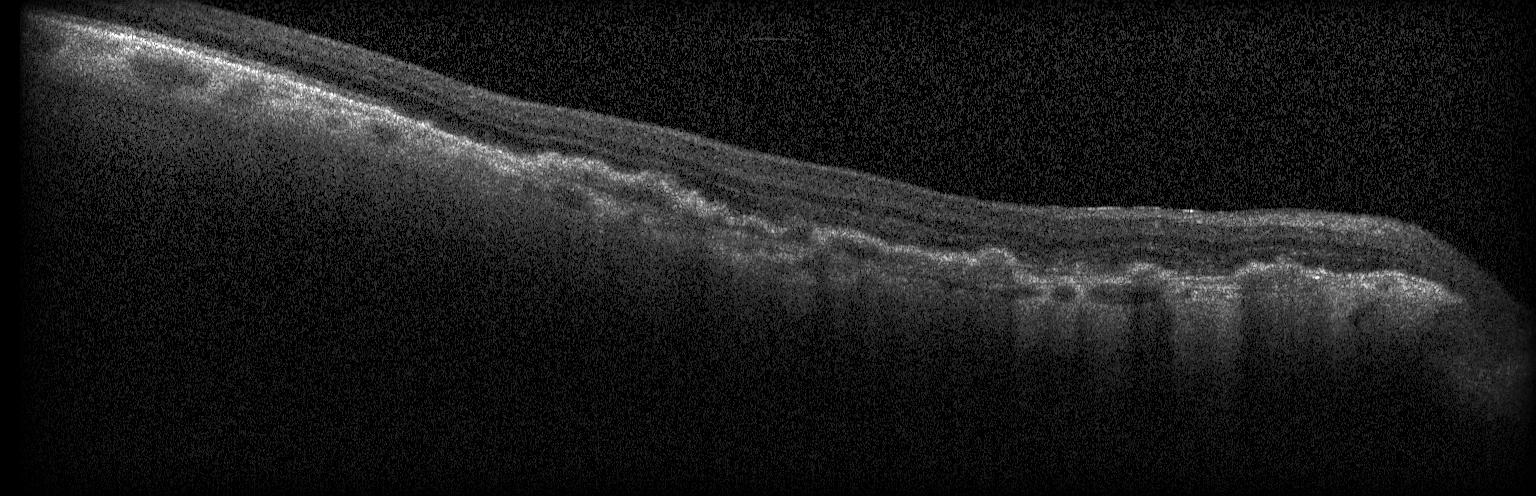

Acquired on a Heidelberg Spectralis · retinal OCT B-scan. Diagnosis: a choroidal neovascular membrane.